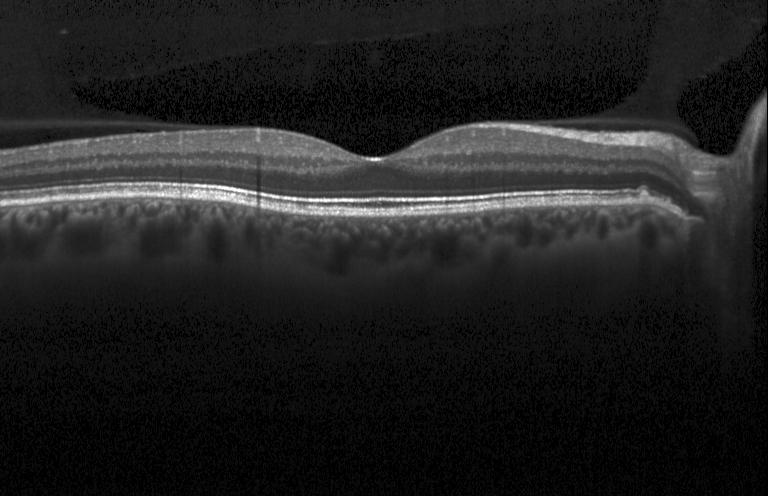

Heidelberg Spectralis. Spectral-domain OCT. OCT B-scan — Assessment: drusen.